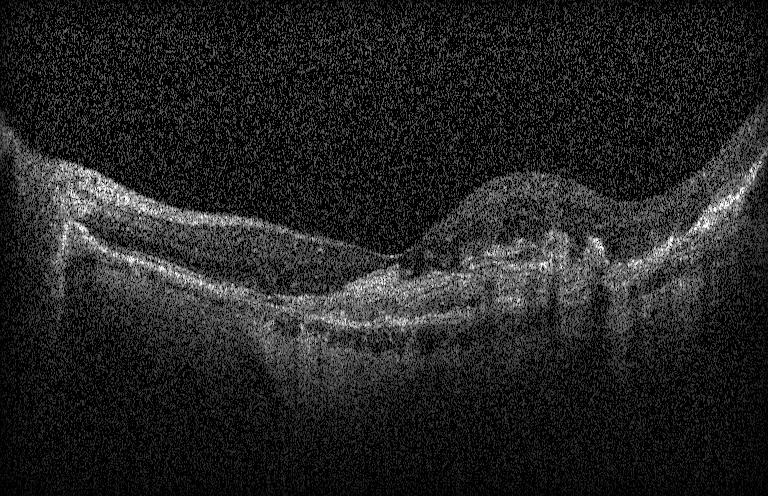 Through the macula · retinal OCT cross-section — Diagnosis: choroidal neovascularization.